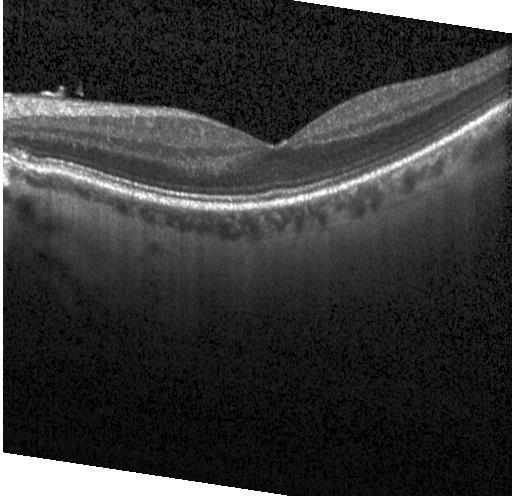
Spectral-domain OCT; OCT line scan.
This B-scan demonstrates no CNV, DME, or drusen.